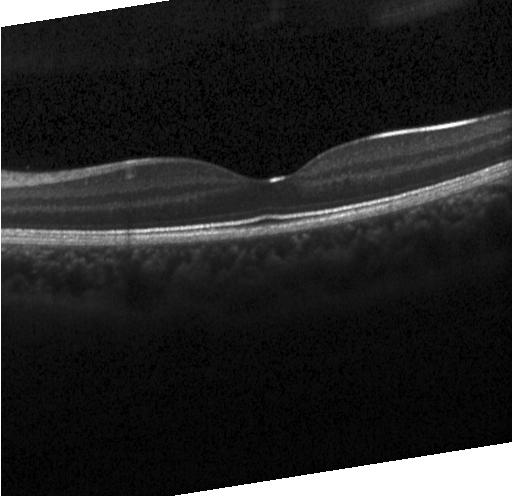

OCT B-scan.
Assessment: no evidence of choroidal neovascularization, diabetic macular edema, or drusen.